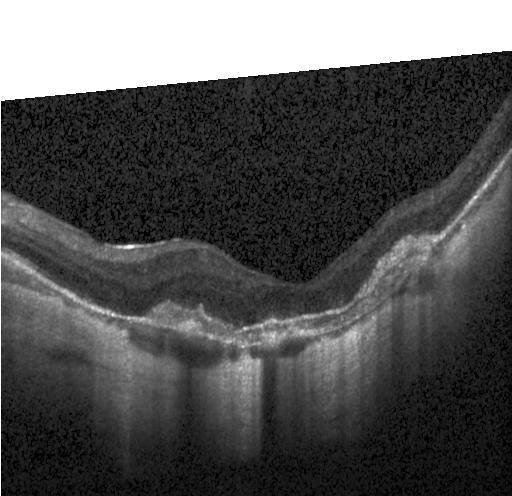

Spectral-domain optical coherence tomography · retinal OCT cross-section · Heidelberg Spectralis
Diagnosis: CNV.